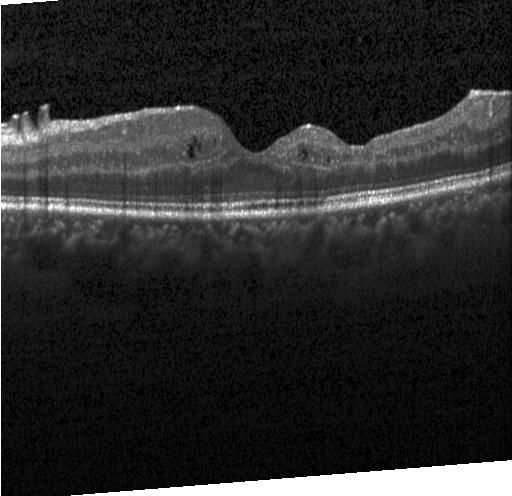 Retinal OCT B-scan, through the macula, acquired on a Heidelberg Spectralis — This B-scan demonstrates diabetic macular edema (DME).